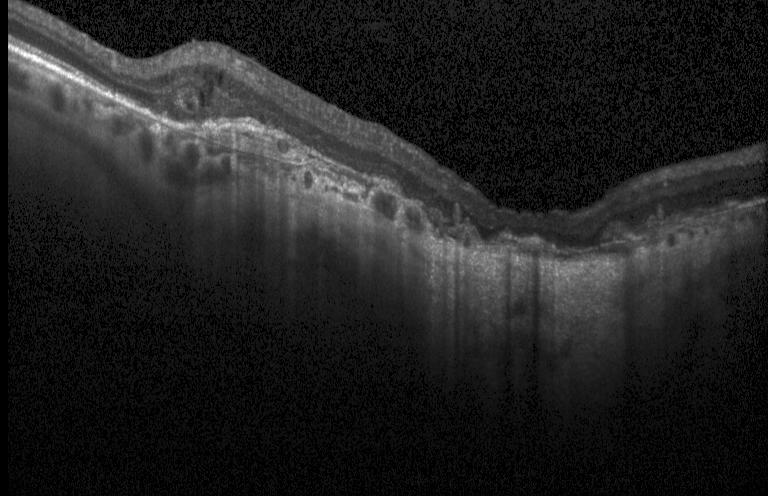
Spectral-domain OCT; OCT line scan.
Finding: choroidal neovascularization.